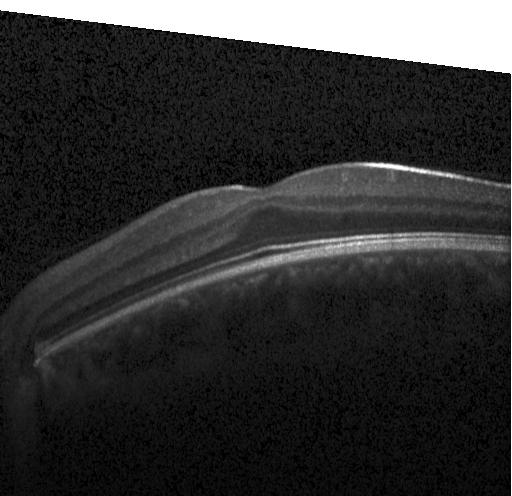
Through the macula. SD-OCT. Optical coherence tomography B-scan. Diagnosis: no choroidal neovascularization, no diabetic macular edema, and no drusen.